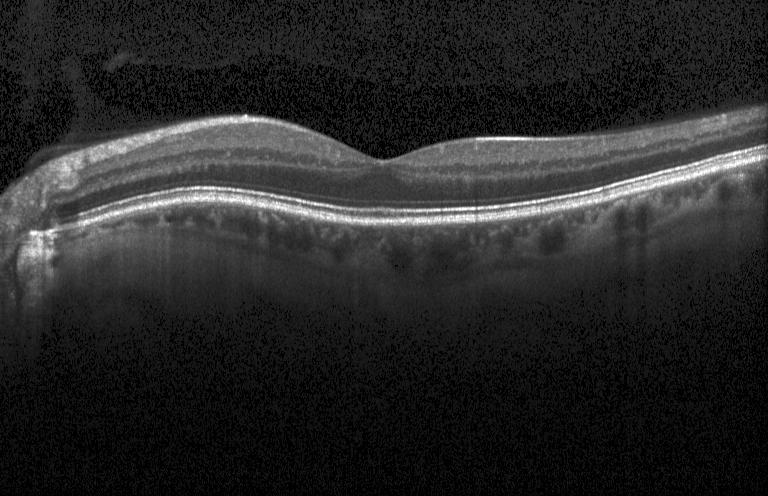

Fovea-centered. Optical coherence tomography scan.
OCT finding: no evidence of choroidal neovascularization, diabetic macular edema, or drusen.